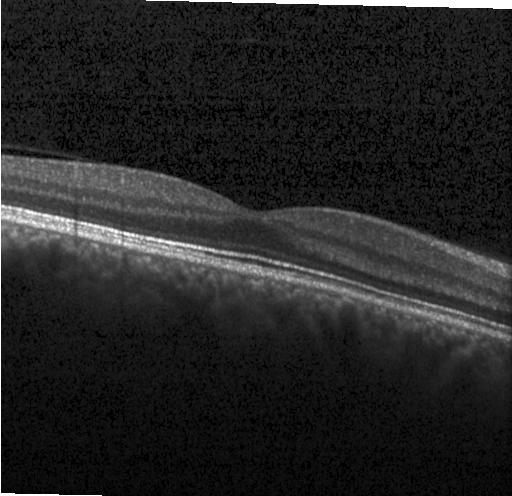

Macular OCT: neither choroidal neovascularization, diabetic macular edema, nor drusen.